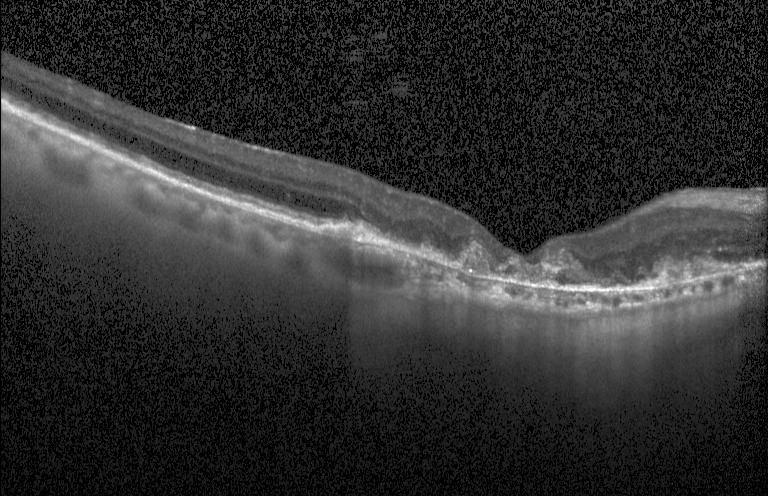

Retinal OCT B-scan, through the macula
Diagnosis: a choroidal neovascular membrane.